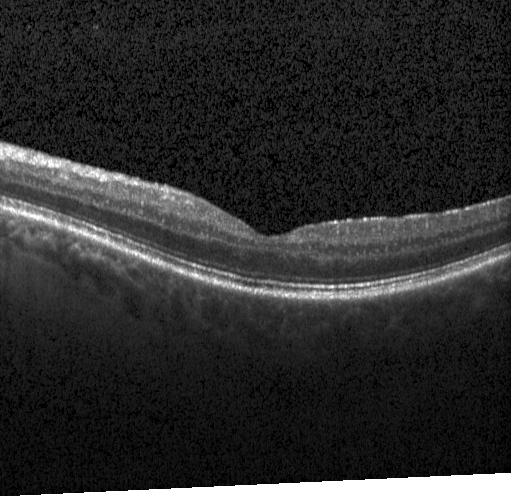
Finding: no choroidal neovascularization, diabetic macular edema, or drusen.